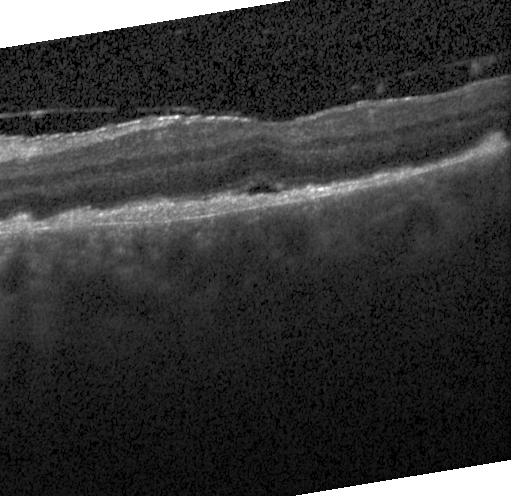 Spectral-domain OCT · optical coherence tomography B-scan · centered on the fovea. Impression: a choroidal neovascular membrane.